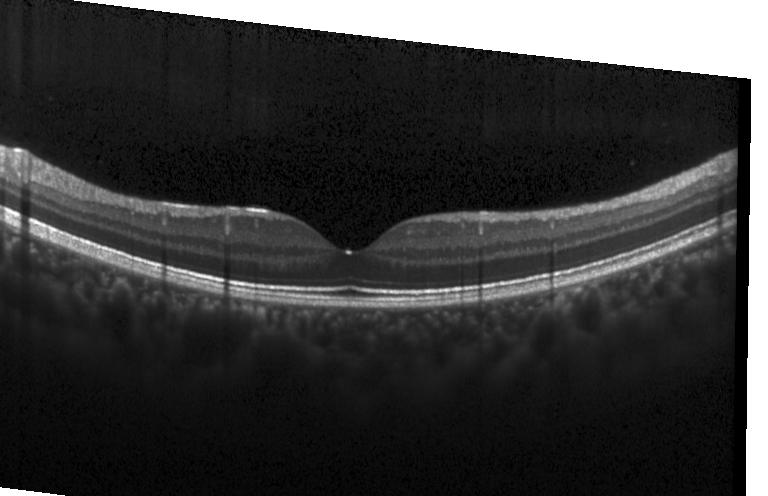

Diagnosis: neither CNV, DME, nor drusen.